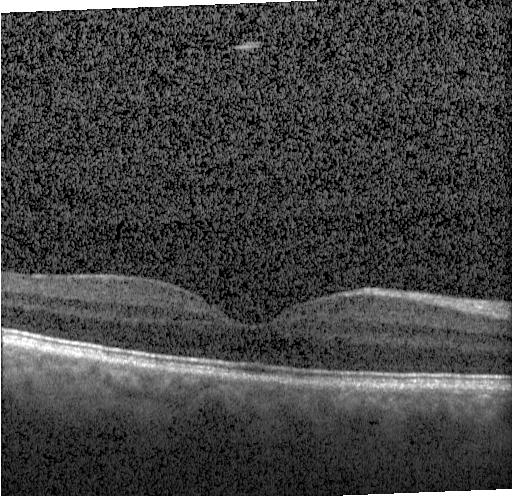 Optical coherence tomography B-scan
OCT finding: no evidence of CNV, DME, or drusen.